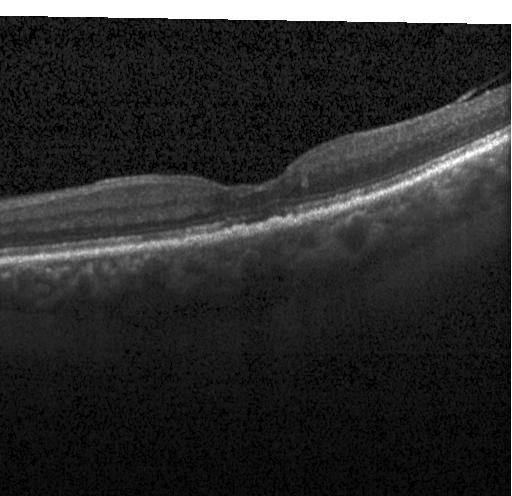

OCT line scan.
This B-scan demonstrates drusen.